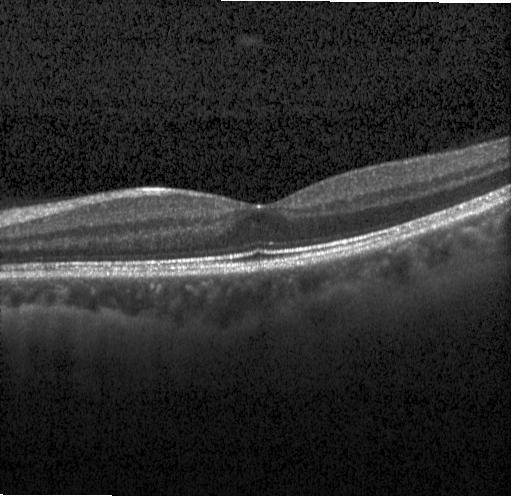

Macular OCT demonstrating no choroidal neovascularization, diabetic macular edema, or drusen.